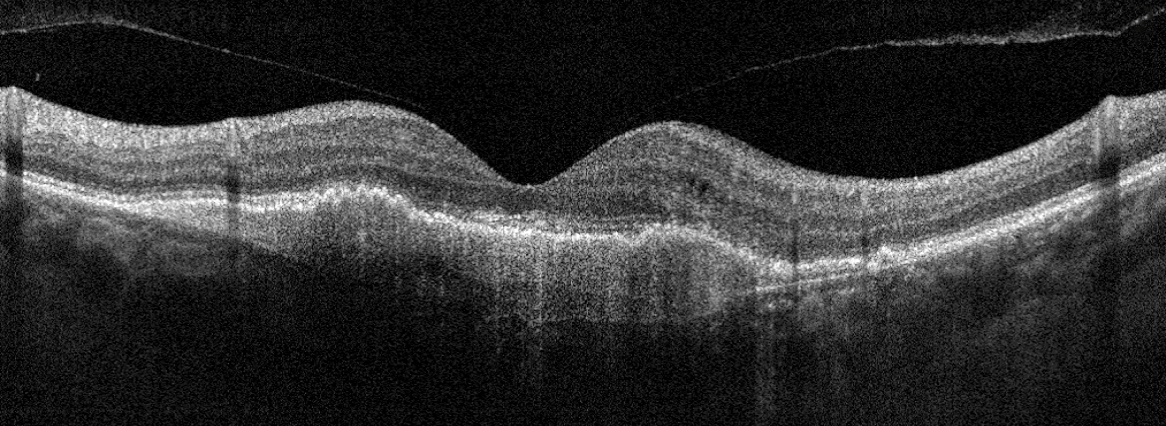 OCT line scan; oculus sinister
Impression: age-related macular degeneration.